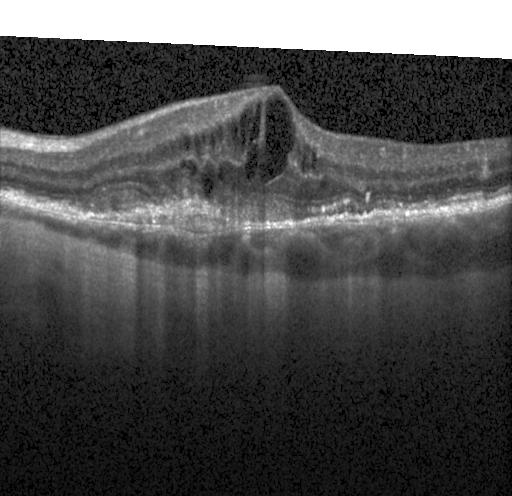
Retinal OCT B-scan; spectral-domain optical coherence tomography.
Diagnosis: CNV.